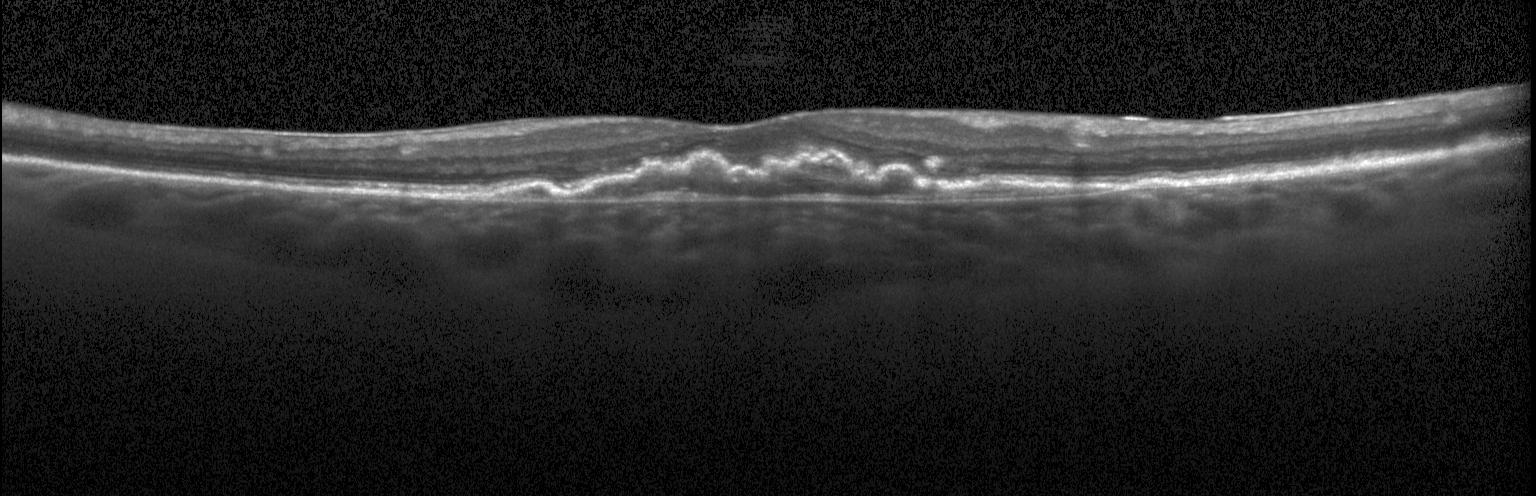

Retinal OCT cross-section showing choroidal neovascularization (CNV).